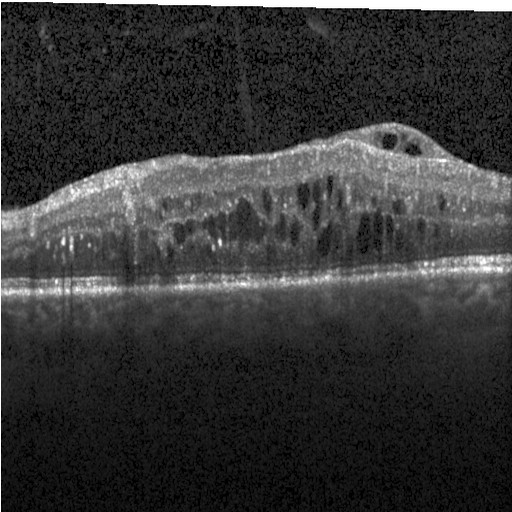

Acquired on a Heidelberg Spectralis, centered on the fovea, optical coherence tomography scan, spectral-domain optical coherence tomography — Impression: diabetic macular edema (DME).